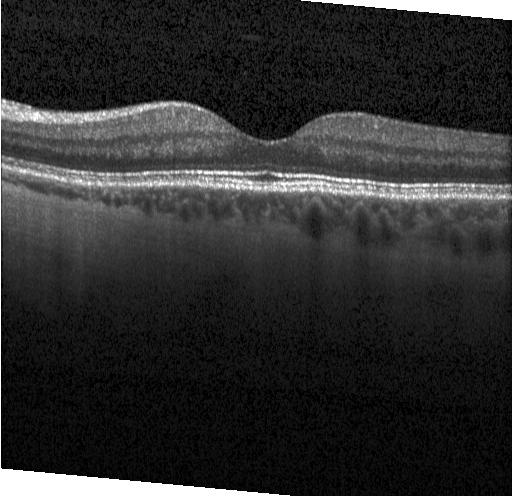

Retinal OCT B-scan. Heidelberg Spectralis OCT system. Through the macula
Diagnosis: neither choroidal neovascularization, diabetic macular edema, nor drusen.